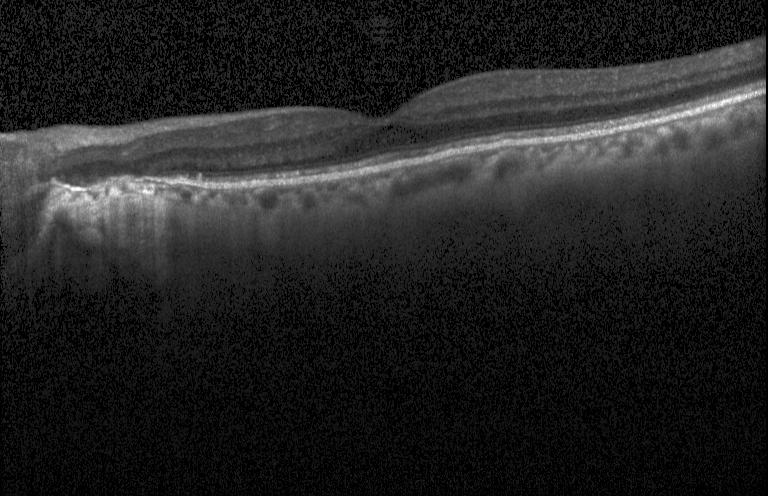 Optical coherence tomography B-scan. Impression: no evidence of CNV, DME, or drusen.